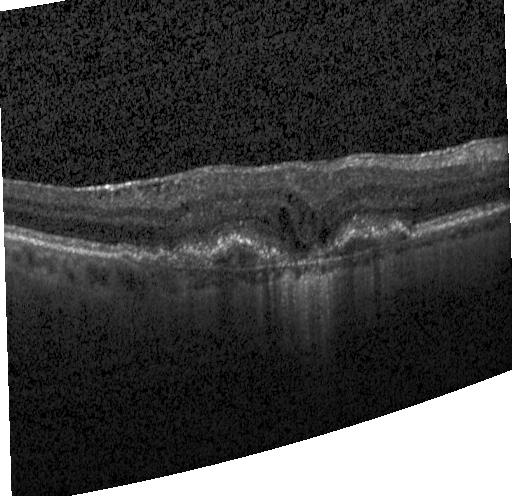

Assessment: choroidal neovascularization.